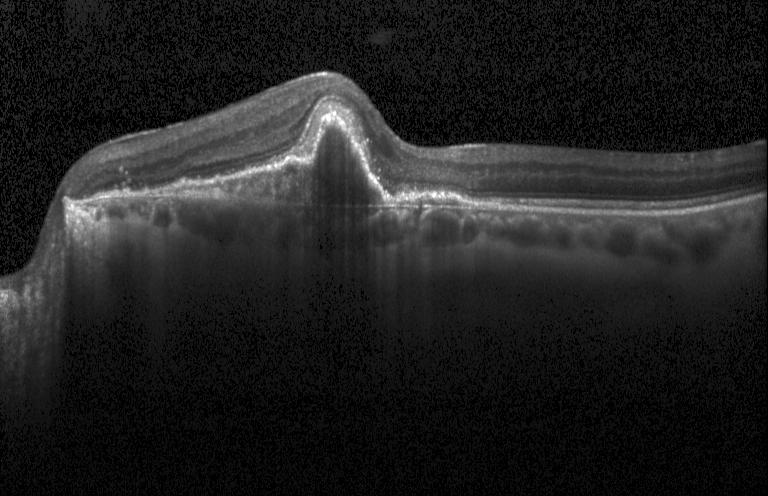

Finding: choroidal neovascularization (CNV).